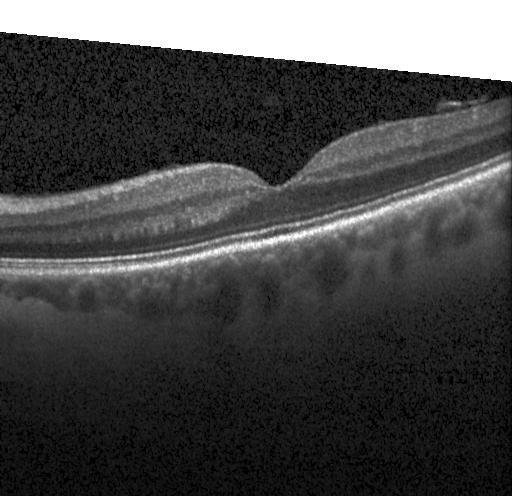

Retinal OCT cross-section
The scan shows no choroidal neovascularization, diabetic macular edema, or drusen.